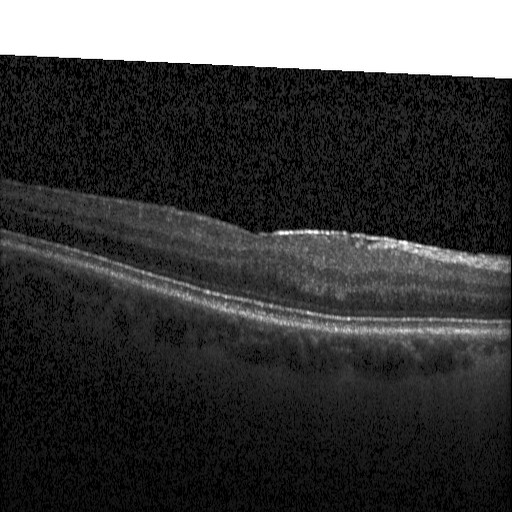 Retinal OCT cross-section. Through the macula. SD-OCT. Heidelberg Spectralis
This B-scan demonstrates diabetic macular edema (DME).